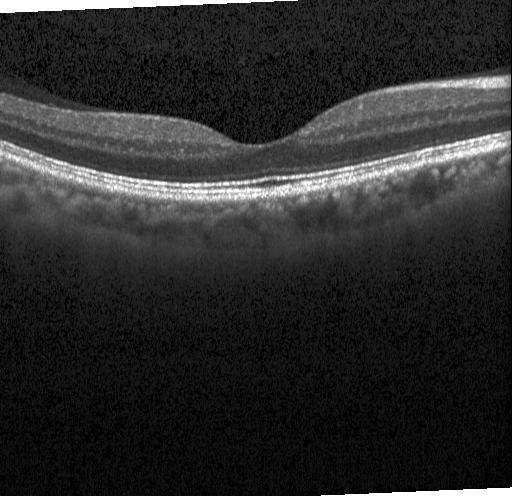
Retinal OCT B-scan, centered on the fovea, acquired on a Heidelberg Spectralis, spectral-domain OCT
The scan shows neither choroidal neovascularization, diabetic macular edema, nor drusen.